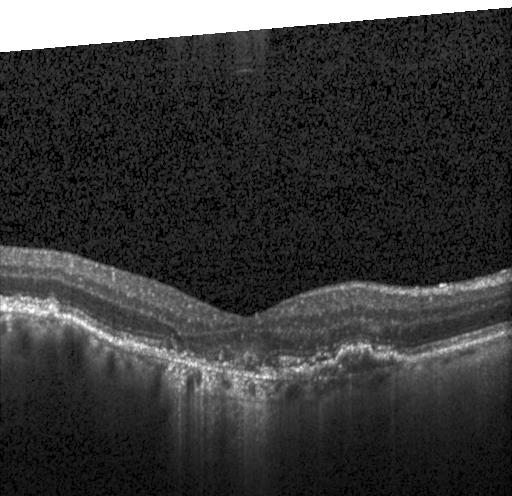
Assessment: CNV.